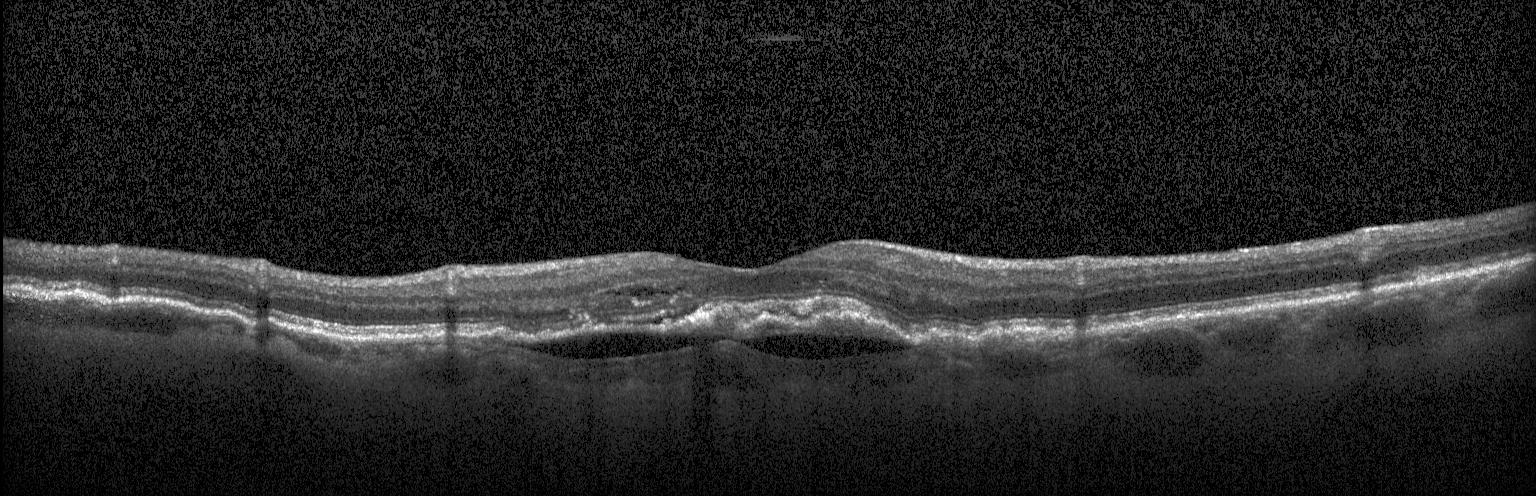

Fovea-centered, spectral-domain OCT, retinal OCT B-scan, acquired on a Heidelberg Spectralis — Impression: a choroidal neovascular membrane.